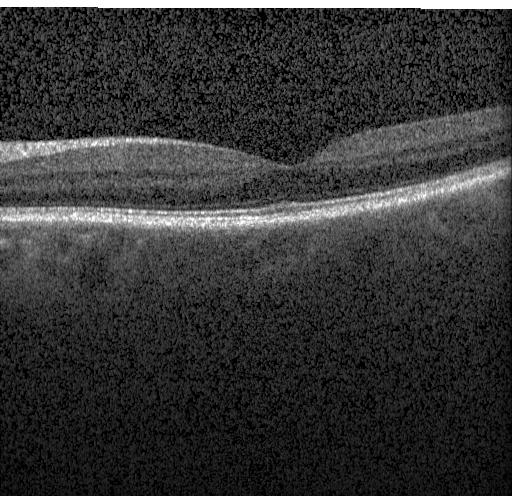
OCT B-scan. SD-OCT
The scan shows no CNV, DME, or drusen.